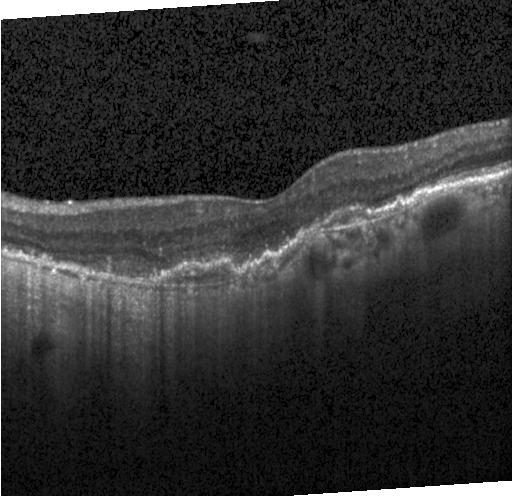 OCT line scan, instrument: Heidelberg Spectralis
Finding: a choroidal neovascular membrane.